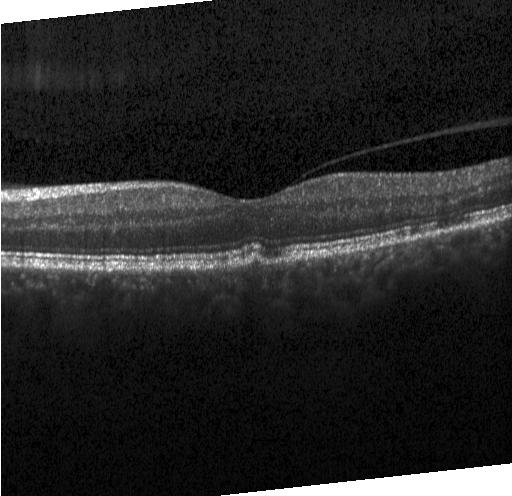

Retinal OCT cross-section. Dx: sub-RPE drusenoid deposits.